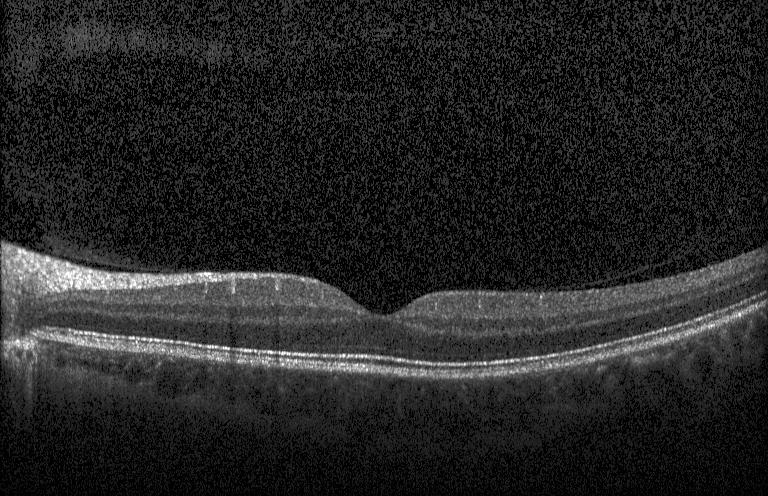
OCT line scan. Fovea-centered. Heidelberg Spectralis.
Finding: neither choroidal neovascularization, diabetic macular edema, nor drusen.